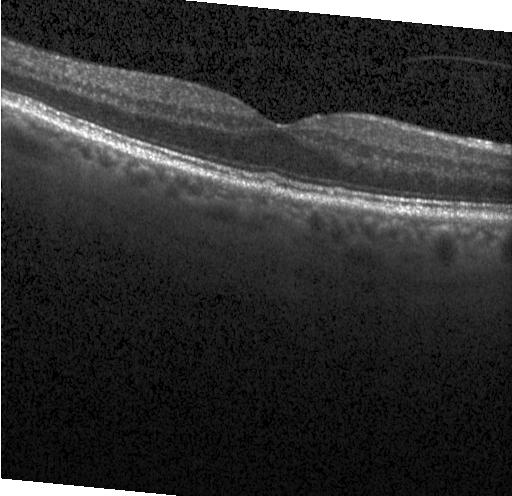
Optical coherence tomography B-scan, instrument: Heidelberg Spectralis — The scan shows no choroidal neovascularization, diabetic macular edema, or drusen.